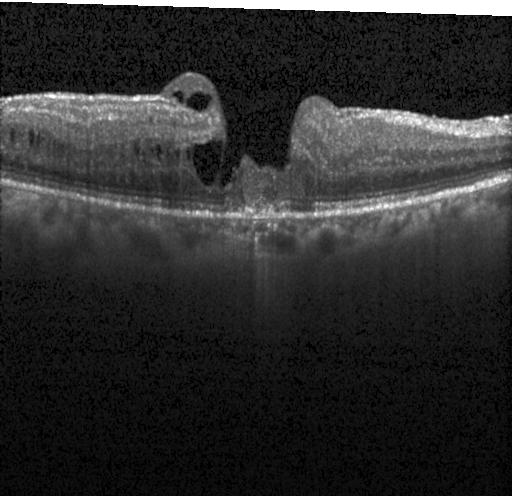 OCT B-scan · Heidelberg Spectralis · SD-OCT · through the macula
Impression: DME.